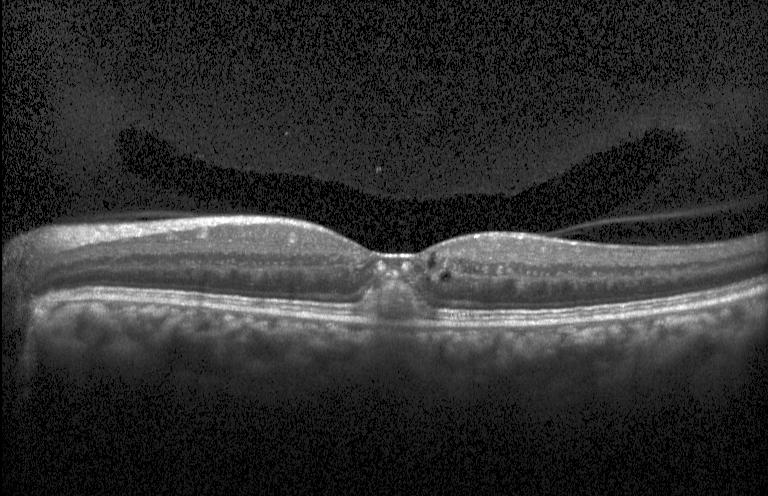 Heidelberg Spectralis OCT system. SD-OCT. OCT B-scan.
Finding: choroidal neovascularization (CNV).